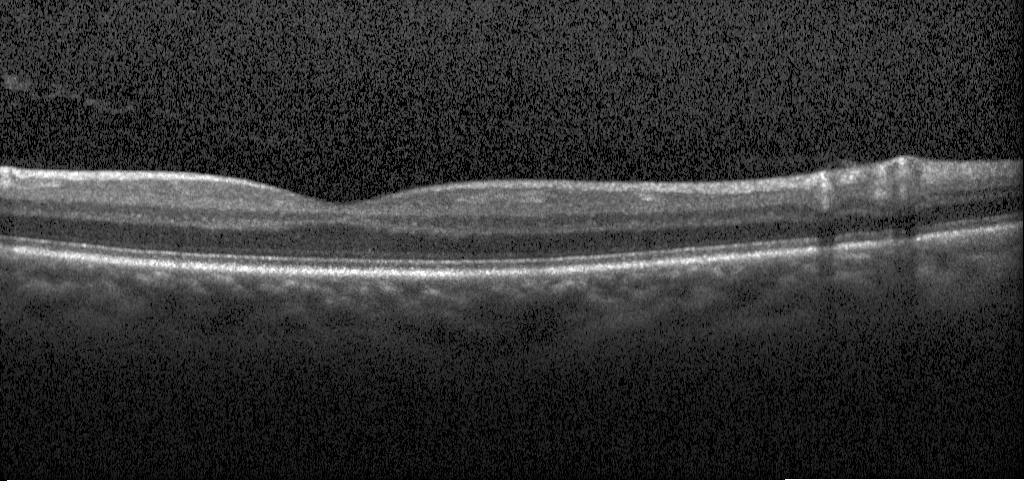 OCT finding: no evidence of CNV, DME, or drusen.